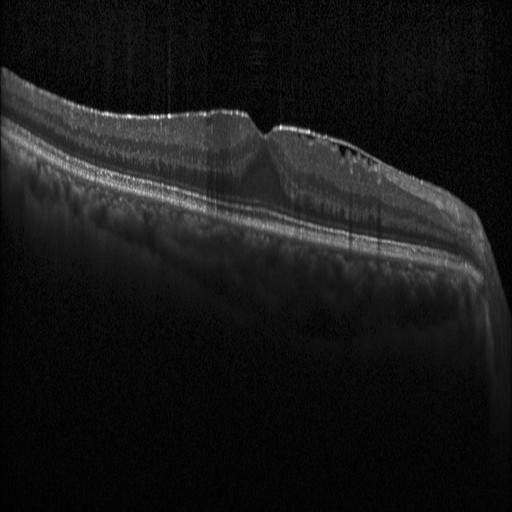
Diagnosis: diabetic macular edema.